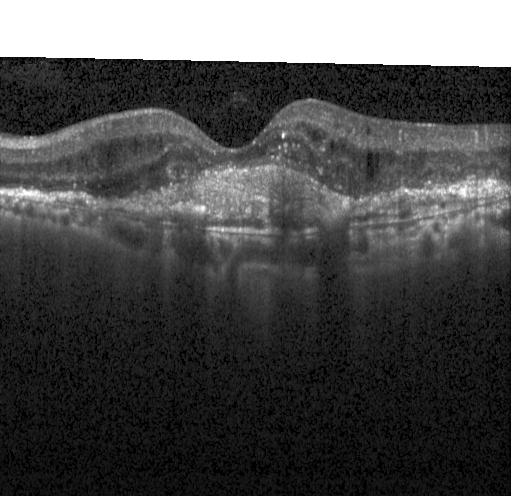
Dx: a choroidal neovascular membrane.